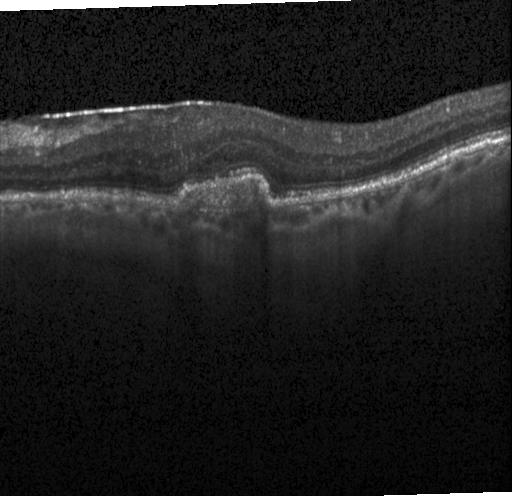

Retinal OCT B-scan. OCT finding: a choroidal neovascular membrane.